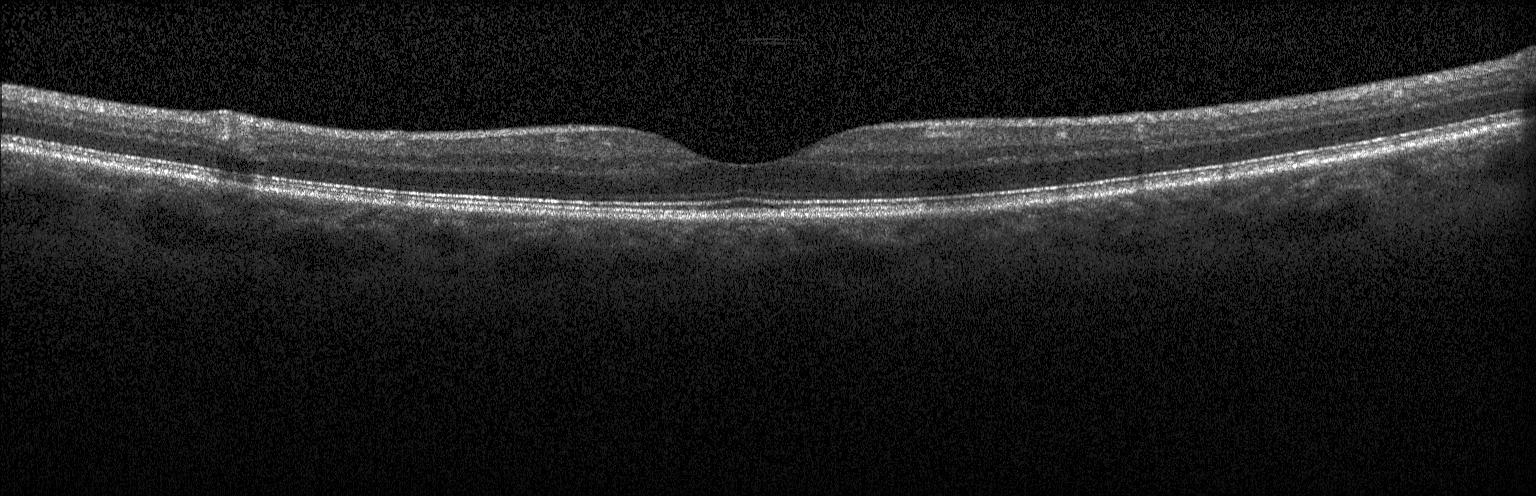
Finding: no CNV, no DME, and no drusen.